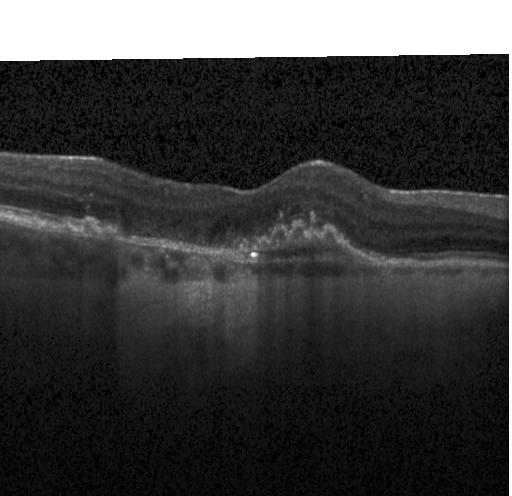 OCT line scan.
Finding: choroidal neovascularization (CNV).